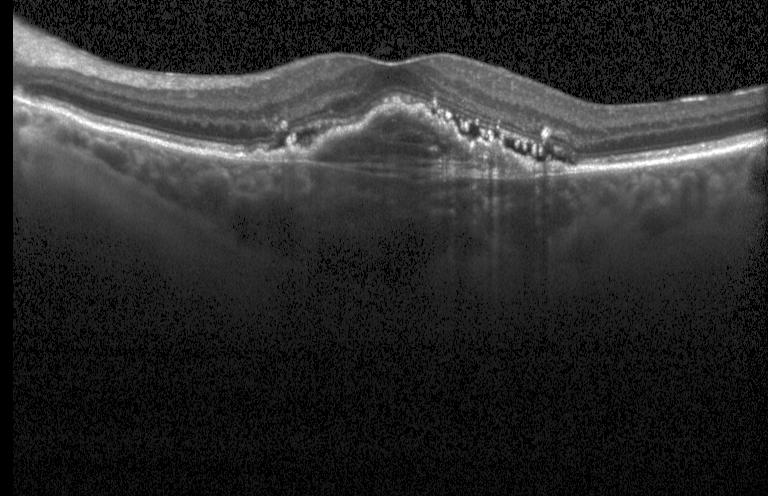
Finding: a choroidal neovascular membrane.